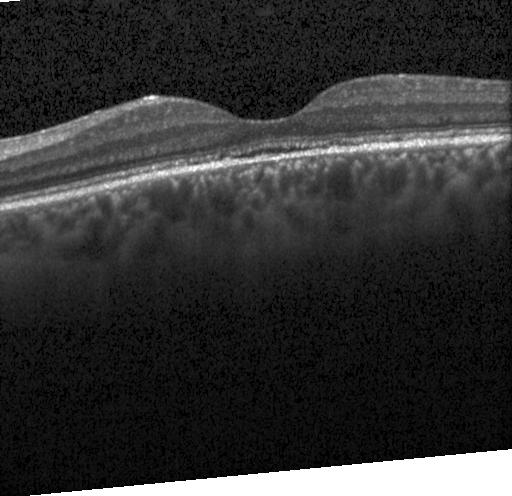 Spectral-domain OCT B-scan: no CNV, no DME, and no drusen.